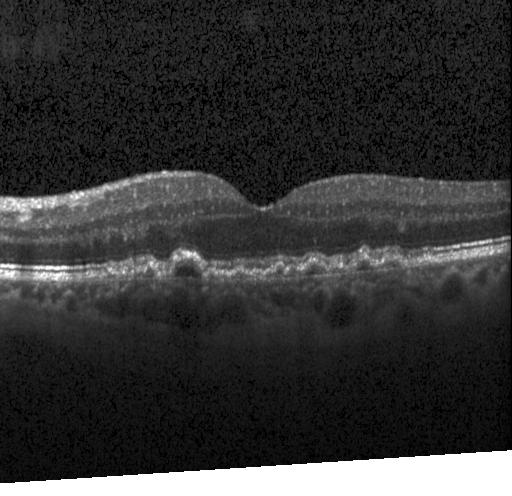 SD-OCT. Horizontal scan through the fovea. OCT line scan. Acquired on a Heidelberg Spectralis.
Finding: multiple drusen.